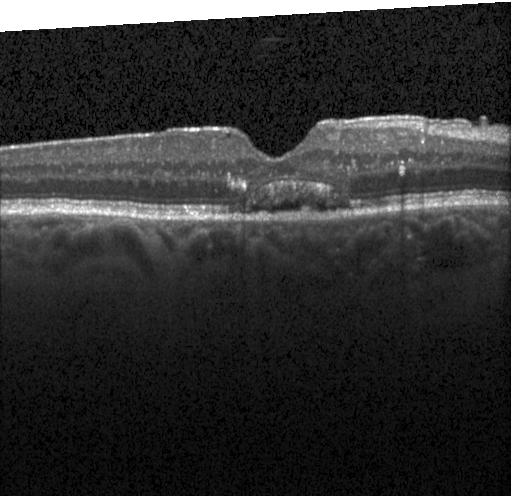
Heidelberg Spectralis · through the macula · OCT B-scan · SD-OCT
Macular OCT: choroidal neovascularization (CNV).